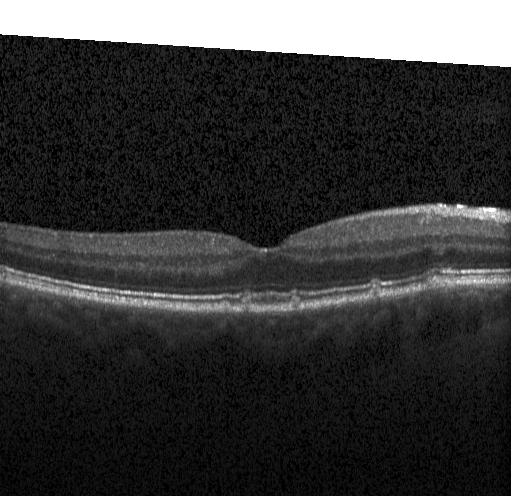
Impression: sub-RPE drusenoid deposits.